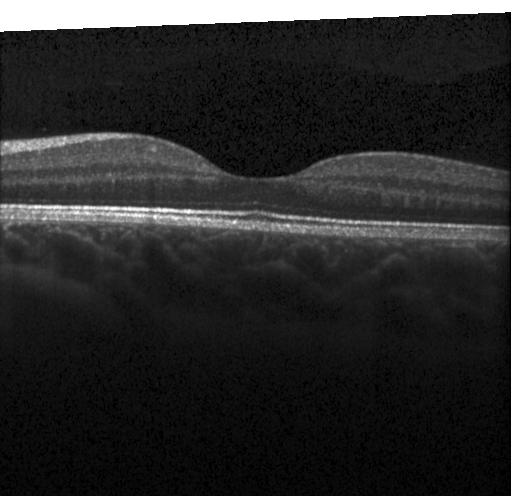
Optical coherence tomography B-scan. Horizontal scan through the fovea. Acquired on a Heidelberg Spectralis. Impression: no evidence of CNV, DME, or drusen.